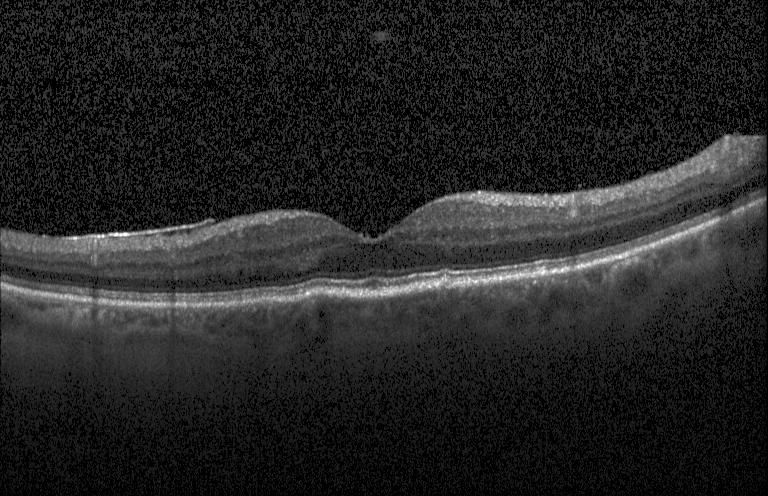
Retinal OCT cross-section — The scan shows sub-RPE drusenoid deposits.